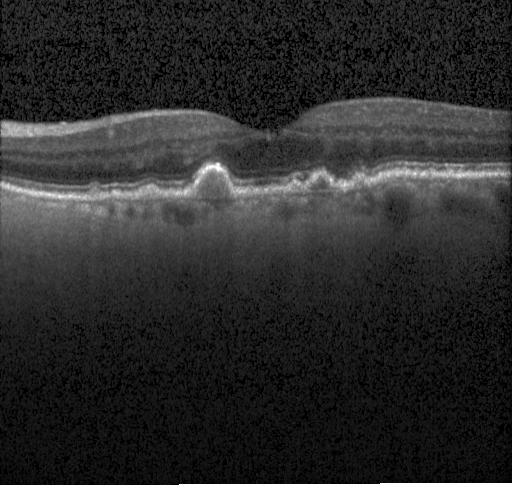 Heidelberg Spectralis, macular scan, optical coherence tomography scan
Finding: sub-RPE drusenoid deposits.